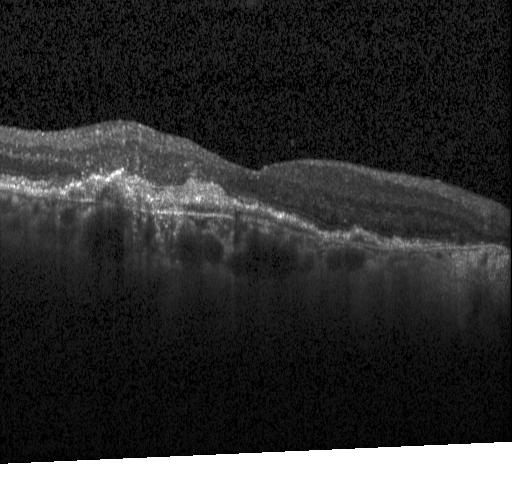

OCT B-scan. This B-scan demonstrates choroidal neovascularization.